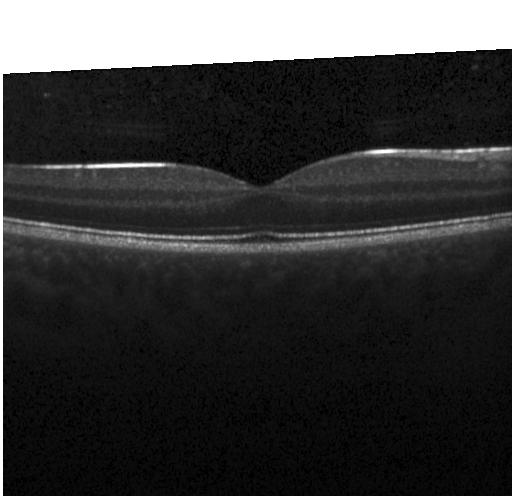
OCT finding: no evidence of choroidal neovascularization, diabetic macular edema, or drusen.